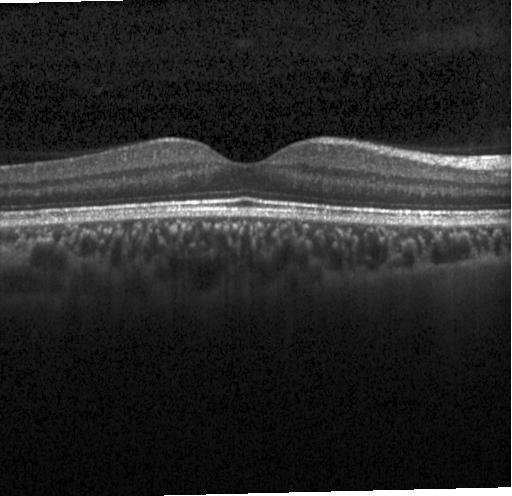 Acquired on a Heidelberg Spectralis. Through the macula. Retinal OCT B-scan. Spectral-domain OCT — The scan shows no evidence of CNV, DME, or drusen.